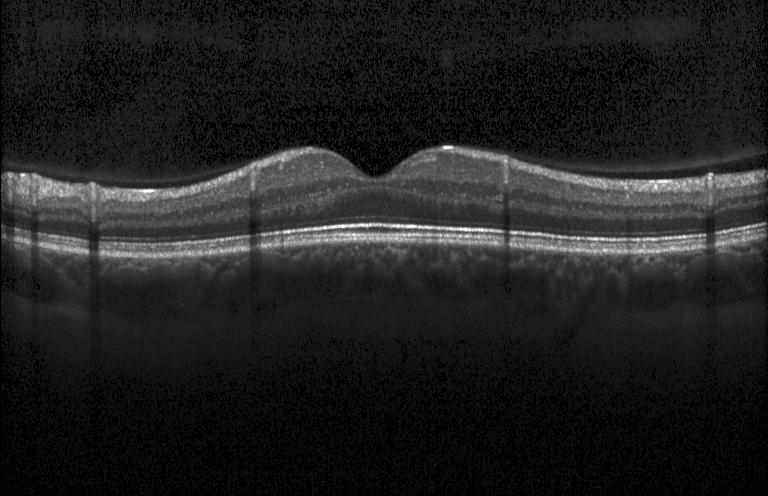
Optical coherence tomography B-scan. No CNV, no DME, and no drusen.